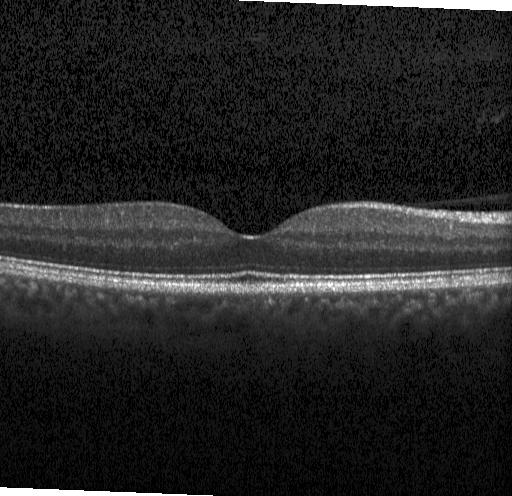
Heidelberg Spectralis; through the macula; retinal OCT cross-section — Impression: no choroidal neovascularization, diabetic macular edema, or drusen.